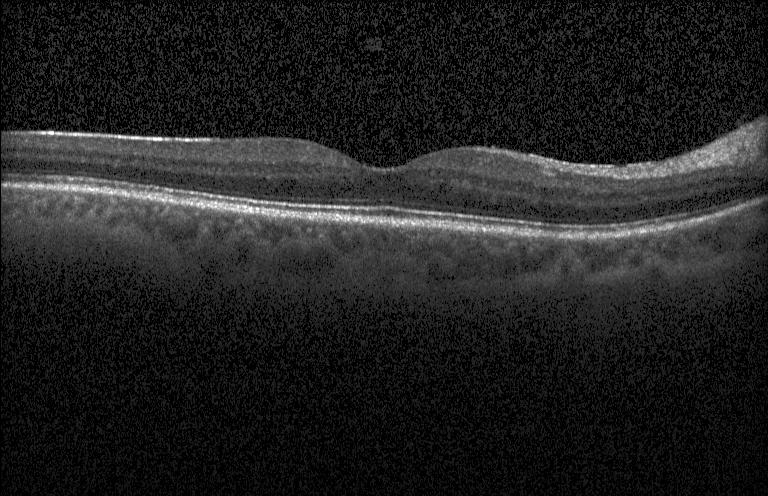 Spectral-domain optical coherence tomography, macular scan, instrument: Heidelberg Spectralis, OCT B-scan
Neither choroidal neovascularization, diabetic macular edema, nor drusen.